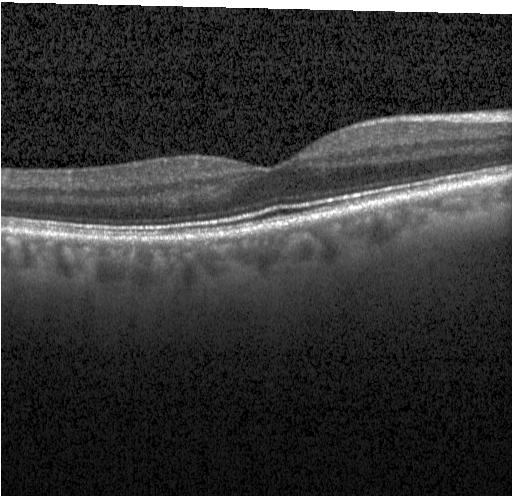
OCT finding: no choroidal neovascularization, no diabetic macular edema, and no drusen.